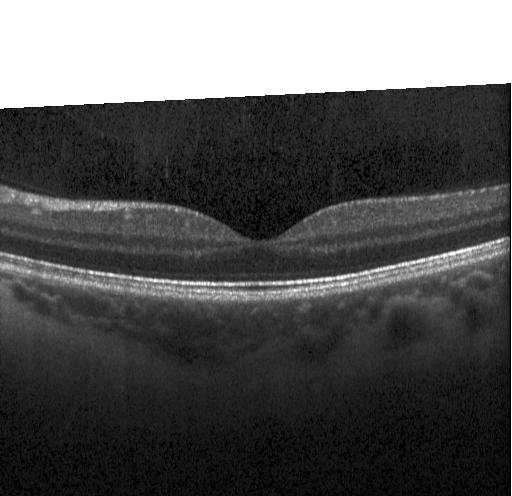 Retinal OCT cross-section.
Assessment: no choroidal neovascularization, diabetic macular edema, or drusen.